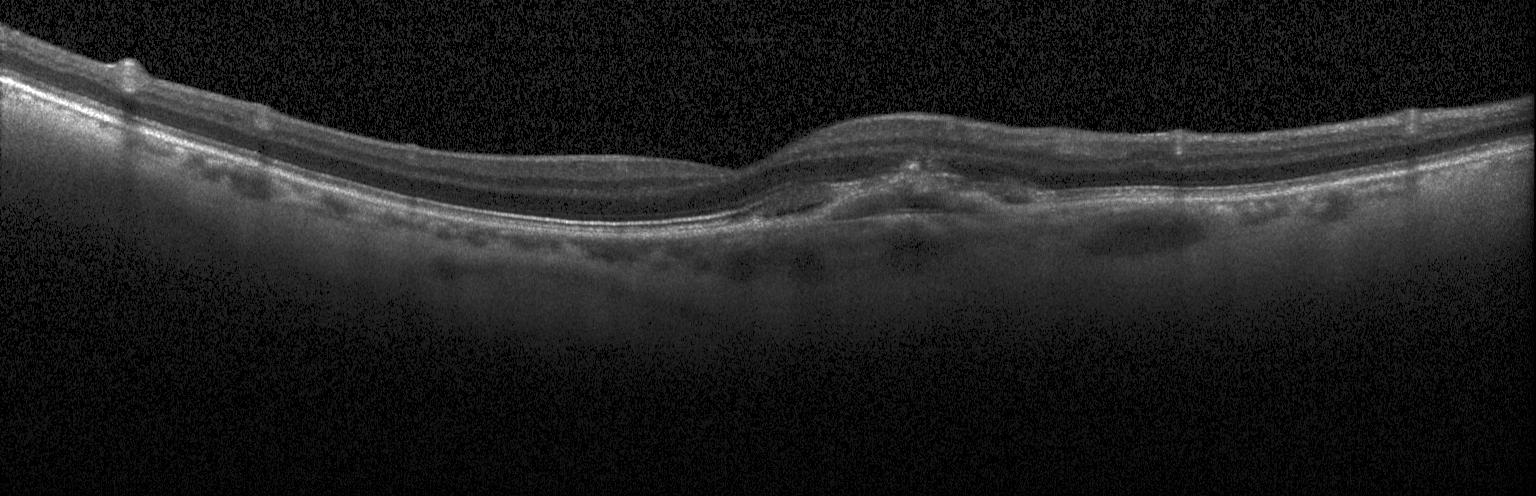

SD-OCT; OCT line scan; acquired on a Heidelberg Spectralis; fovea-centered. This B-scan demonstrates a choroidal neovascular membrane.